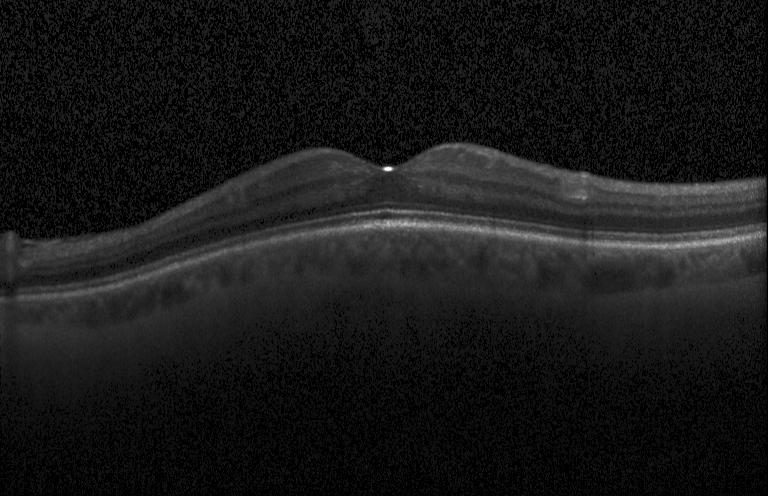 No CNV, DME, or drusen.